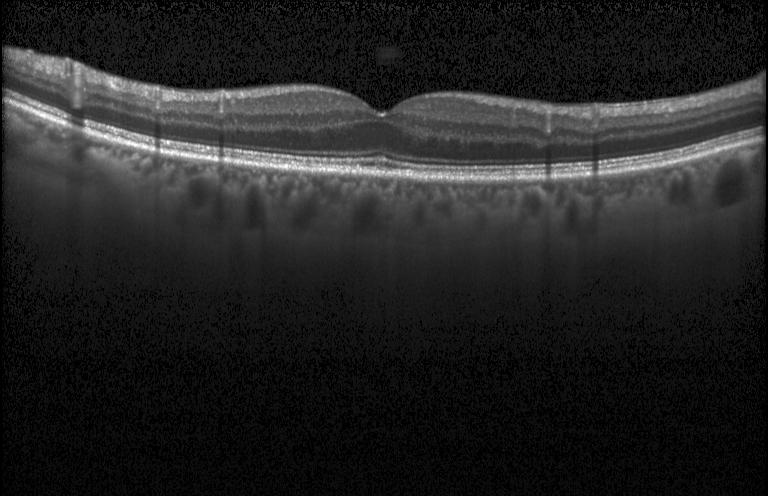 Retinal OCT cross-section, fovea-centered, acquired on a Heidelberg Spectralis
Neither choroidal neovascularization, diabetic macular edema, nor drusen.